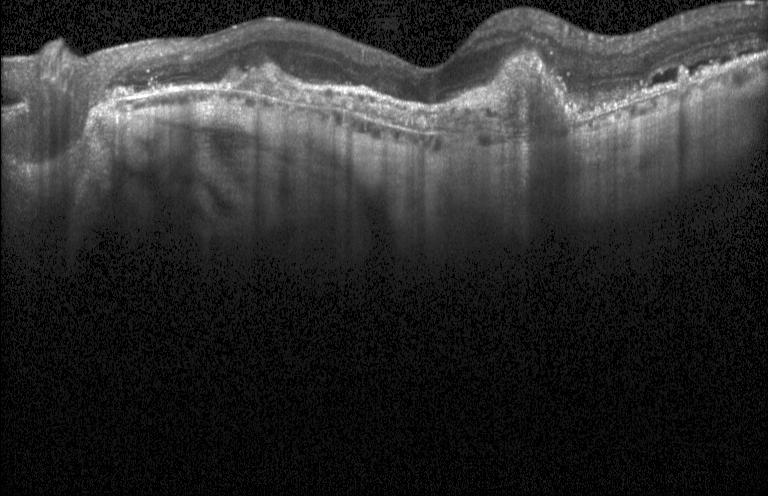

Impression: choroidal neovascularization.